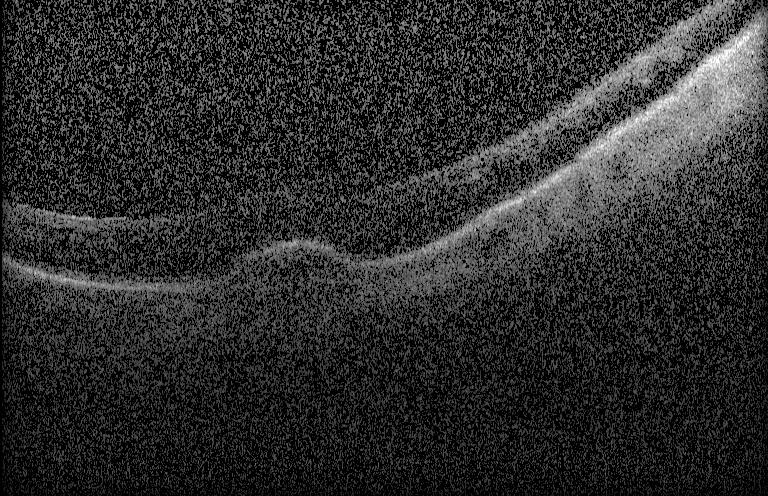 Dx: a choroidal neovascular membrane.